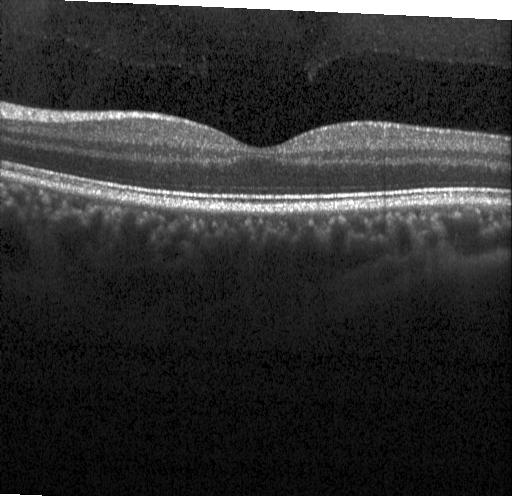

SD-OCT. Optical coherence tomography scan. Fovea-centered. Assessment: no evidence of choroidal neovascularization, diabetic macular edema, or drusen.